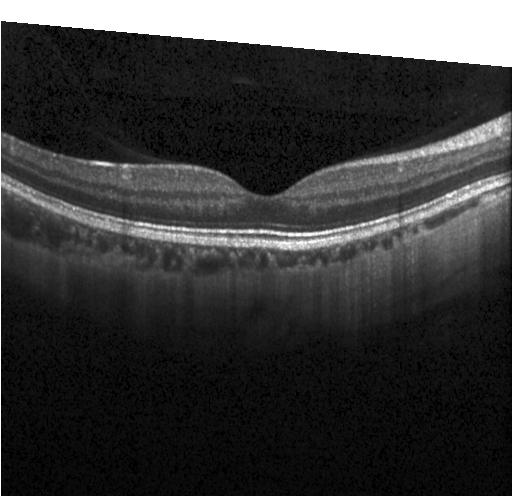
OCT finding: no CNV, DME, or drusen.